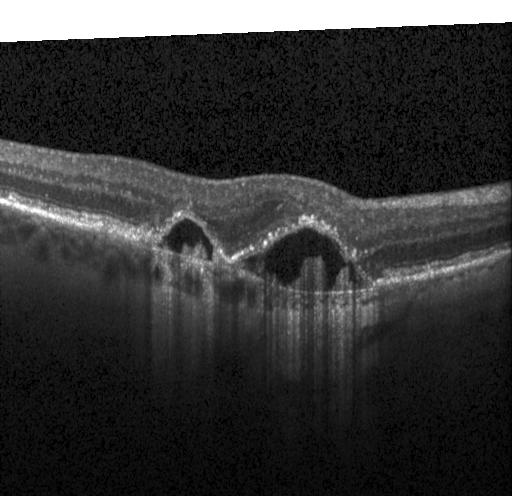

Spectral-domain OCT. Optical coherence tomography scan. Instrument: Heidelberg Spectralis.
The scan shows choroidal neovascularization.